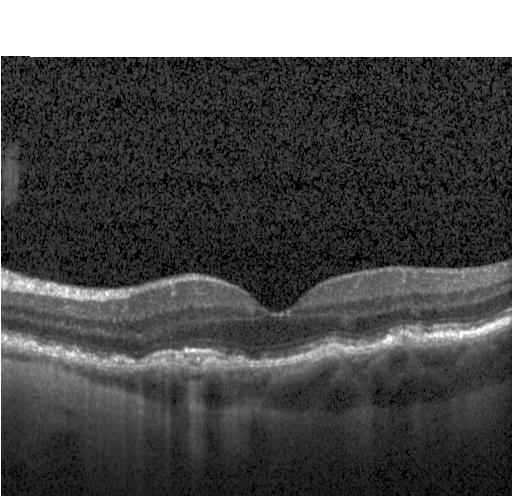 Dx: a choroidal neovascular membrane.